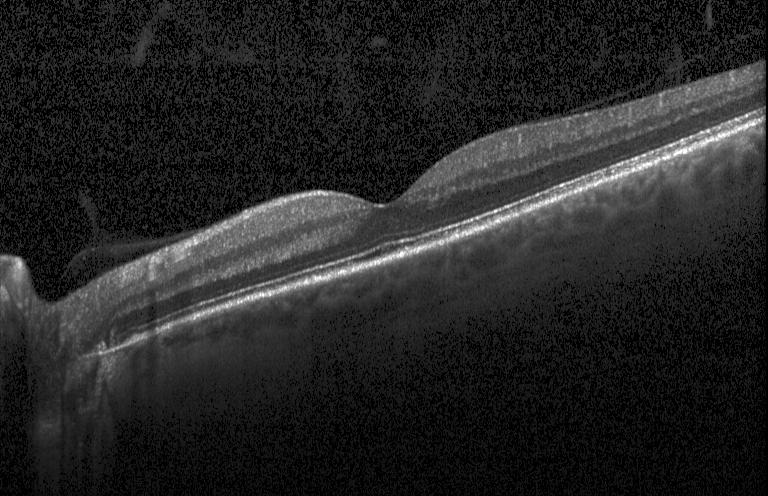
Spectral-domain OCT B-scan: no evidence of choroidal neovascularization, diabetic macular edema, or drusen.